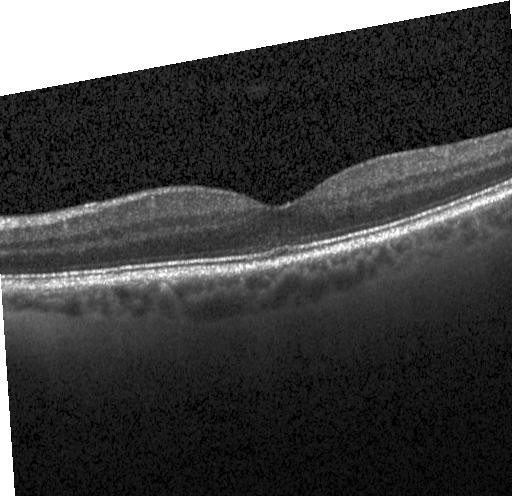 OCT B-scan
Finding: neither CNV, DME, nor drusen.